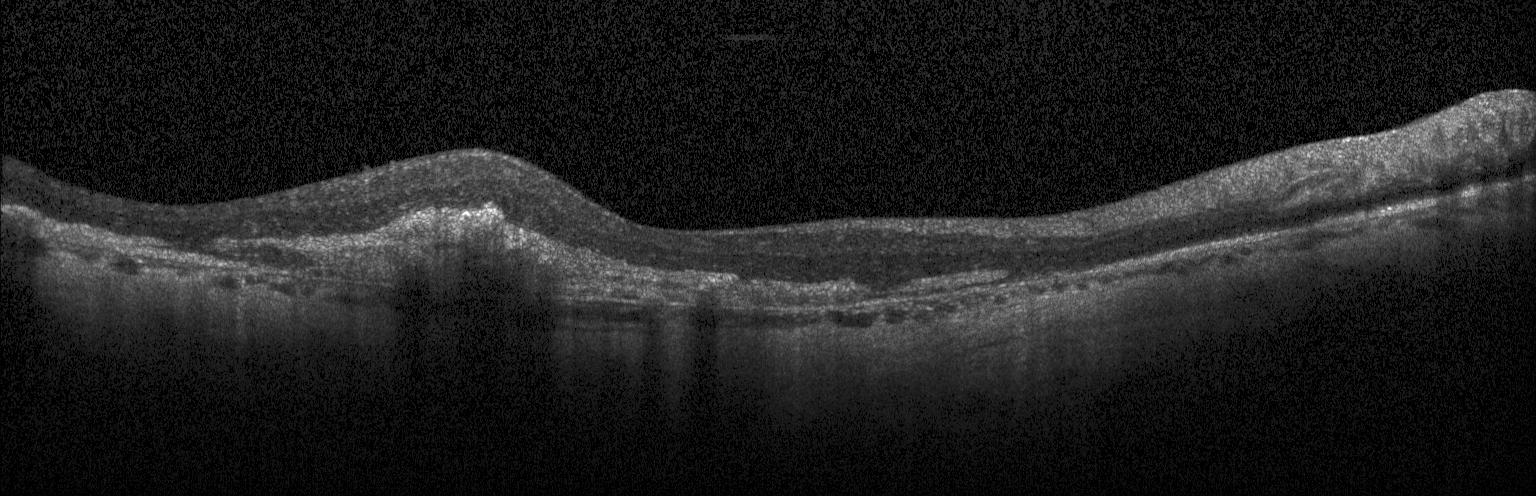

OCT B-scan showing CNV.